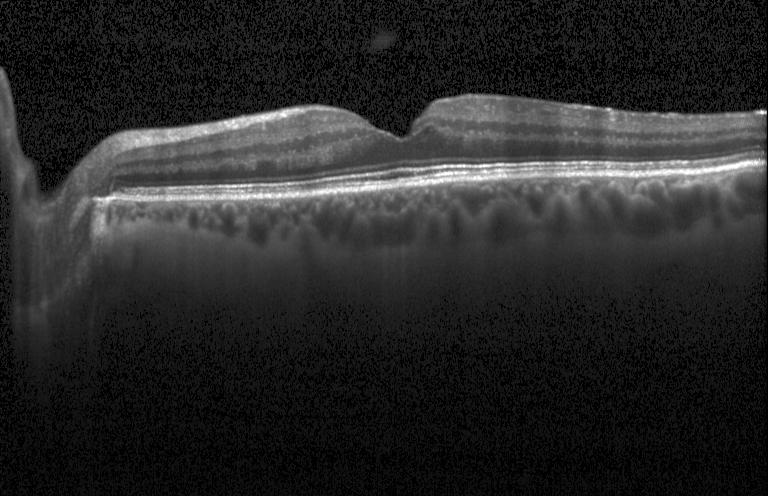 Impression: no choroidal neovascularization, diabetic macular edema, or drusen.